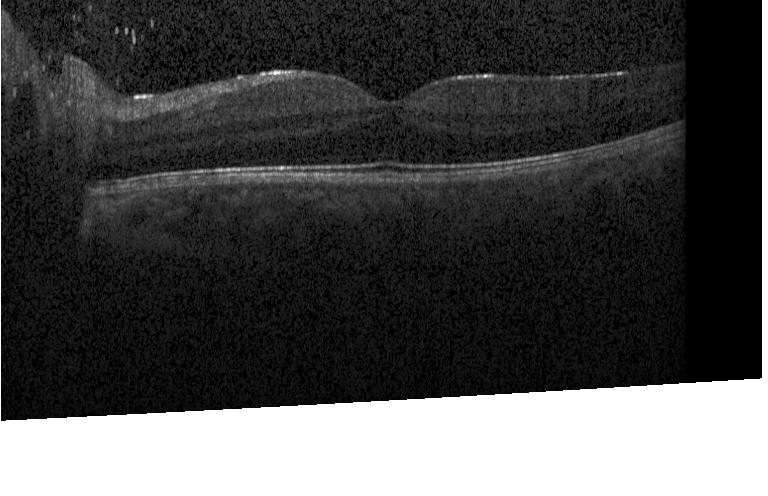
Retinal OCT cross-section showing neither choroidal neovascularization, diabetic macular edema, nor drusen.